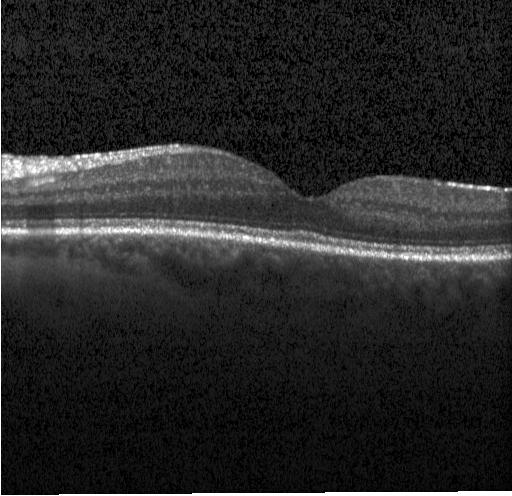

Macular OCT: neither choroidal neovascularization, diabetic macular edema, nor drusen.